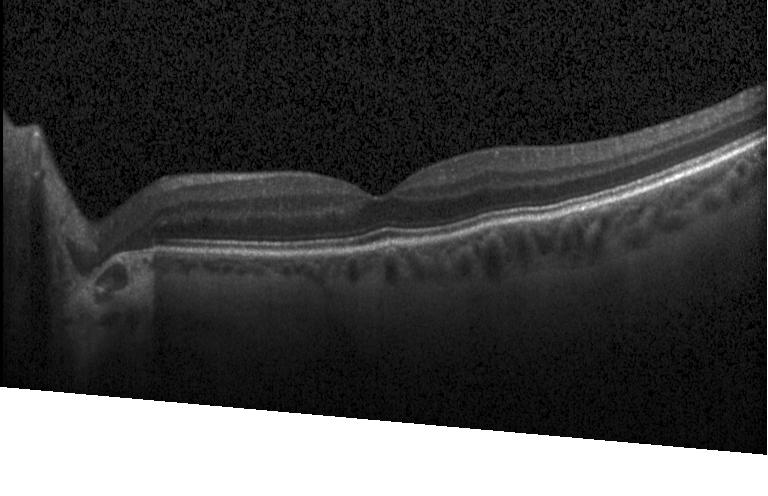

OCT finding: neither choroidal neovascularization, diabetic macular edema, nor drusen.